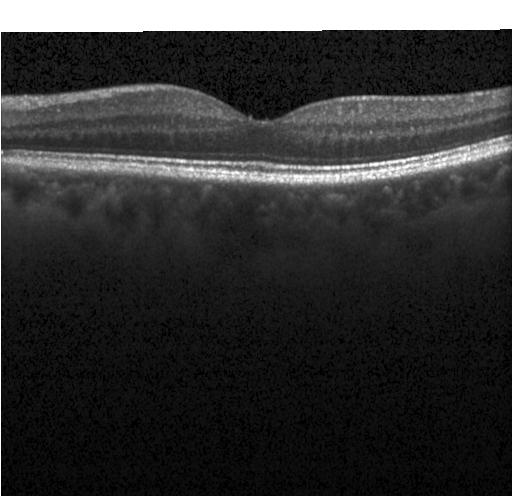 Acquired on a Heidelberg Spectralis · optical coherence tomography scan — Impression: no evidence of choroidal neovascularization, diabetic macular edema, or drusen.